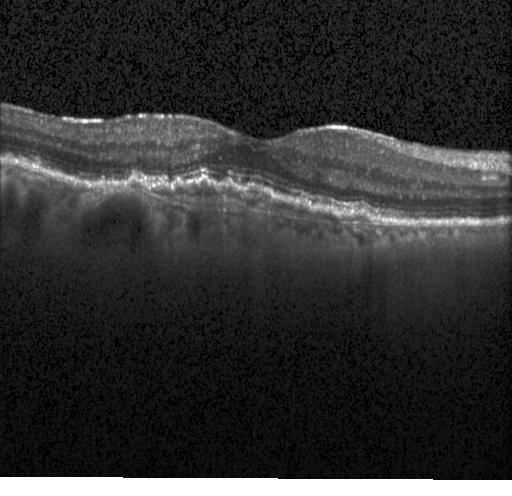

Optical coherence tomography scan. Heidelberg Spectralis OCT system. Fovea-centered. Spectral-domain OCT — A choroidal neovascular membrane.